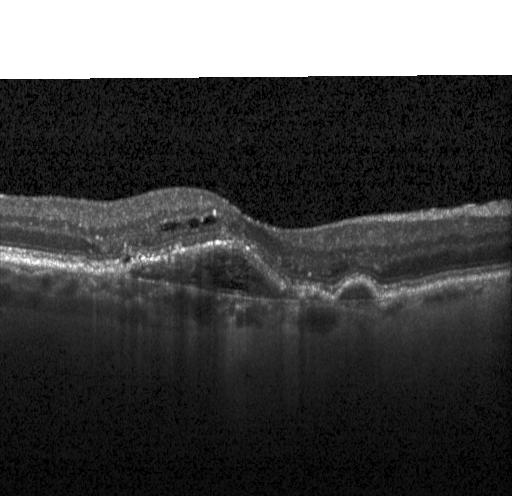
Impression: a choroidal neovascular membrane.